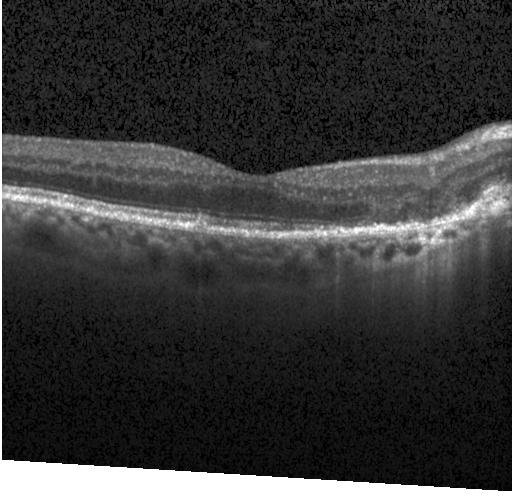 Heidelberg Spectralis, OCT B-scan, macular scan — This B-scan demonstrates choroidal neovascularization.